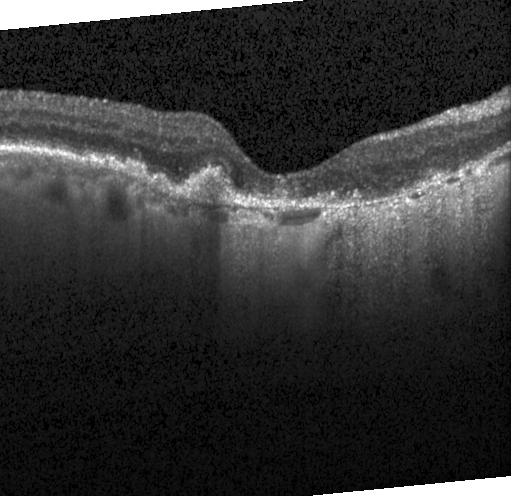

Impression: a choroidal neovascular membrane.